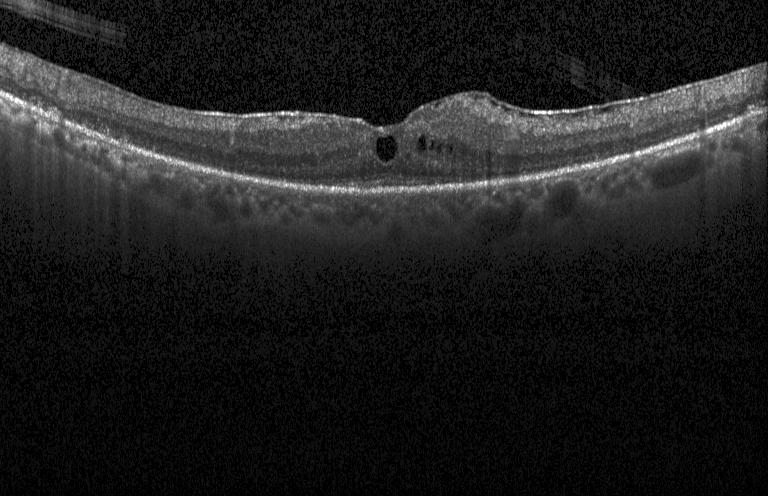 OCT line scan; instrument: Heidelberg Spectralis; spectral-domain optical coherence tomography — This B-scan demonstrates diabetic macular edema (DME).